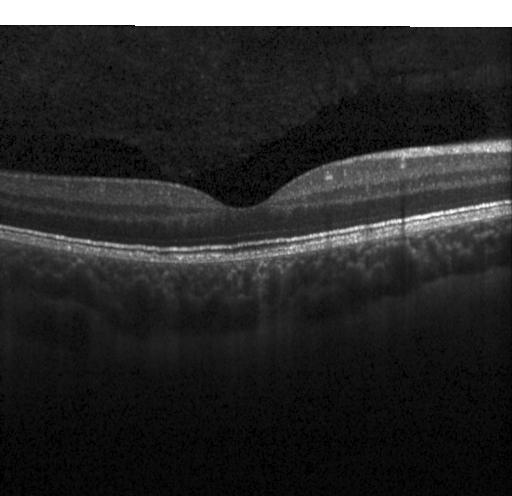

OCT B-scan, centered on the fovea
Impression: no choroidal neovascularization, no diabetic macular edema, and no drusen.